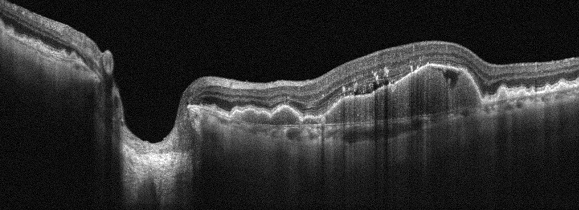 OCT B-scan showing AMD.